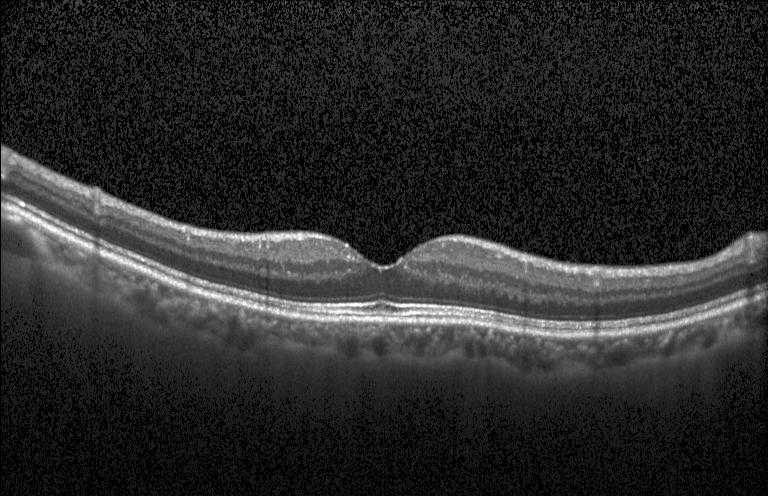 This B-scan demonstrates no CNV, DME, or drusen.